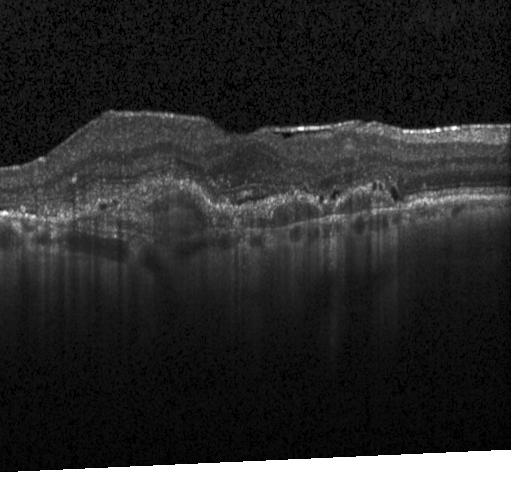

Spectral-domain OCT · OCT B-scan — Macular OCT: CNV.